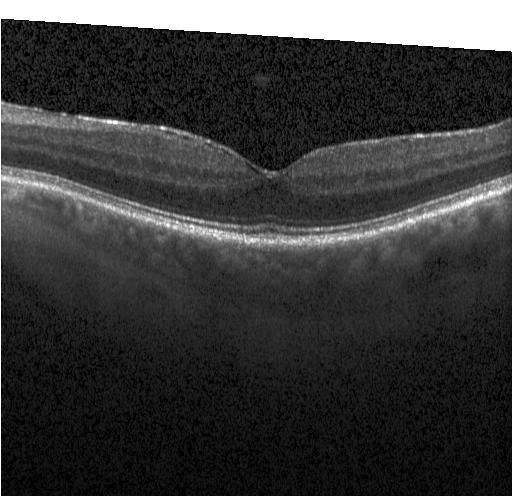

Horizontal scan through the fovea. Retinal OCT B-scan
Assessment: no evidence of choroidal neovascularization, diabetic macular edema, or drusen.